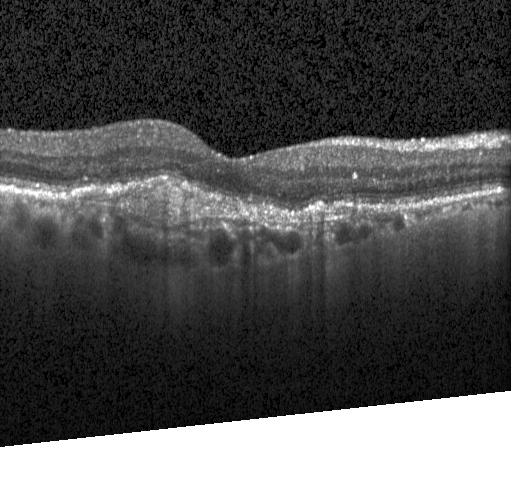
OCT B-scan showing choroidal neovascularization.